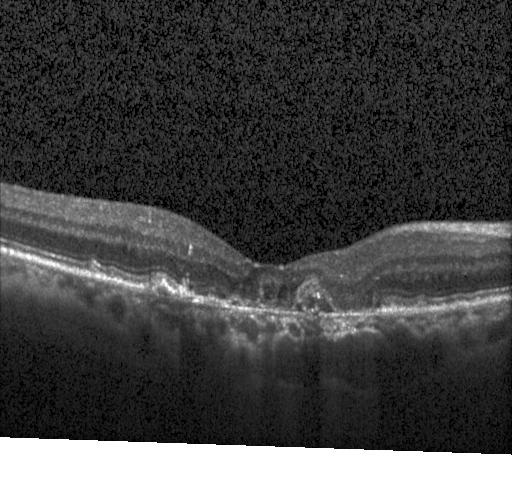

Retinal OCT B-scan · SD-OCT · centered on the fovea — Choroidal neovascularization.